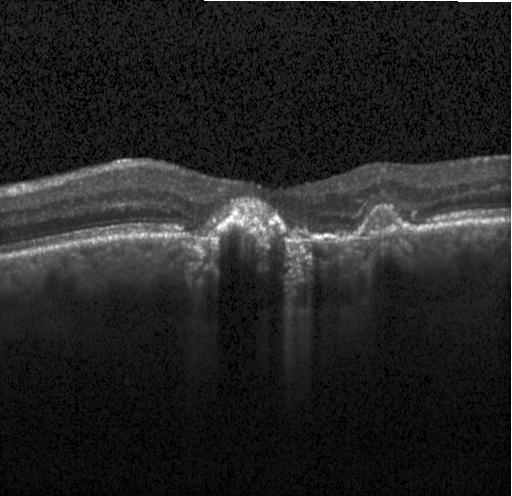

OCT line scan — This B-scan demonstrates a choroidal neovascular membrane.